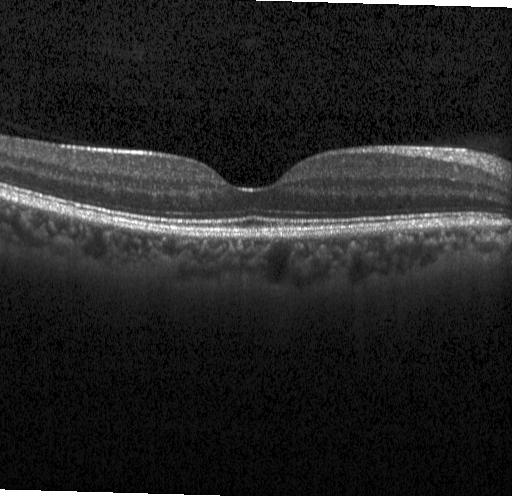

Fovea-centered, retinal OCT cross-section, instrument: Heidelberg Spectralis, SD-OCT. Finding: no choroidal neovascularization, no diabetic macular edema, and no drusen.